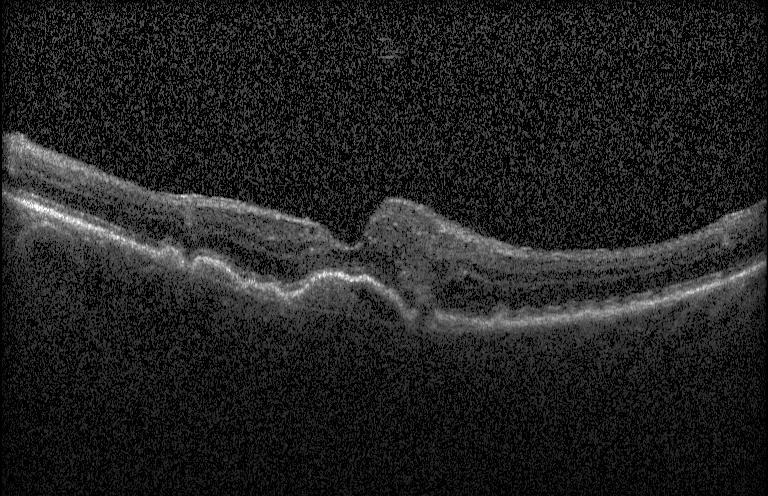

Instrument: Heidelberg Spectralis. OCT line scan. SD-OCT — OCT finding: CNV.